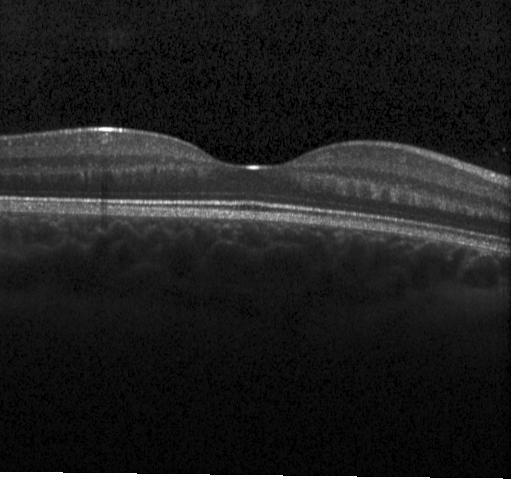

Spectral-domain OCT · horizontal scan through the fovea · optical coherence tomography B-scan · Heidelberg Spectralis — This B-scan demonstrates no choroidal neovascularization, diabetic macular edema, or drusen.